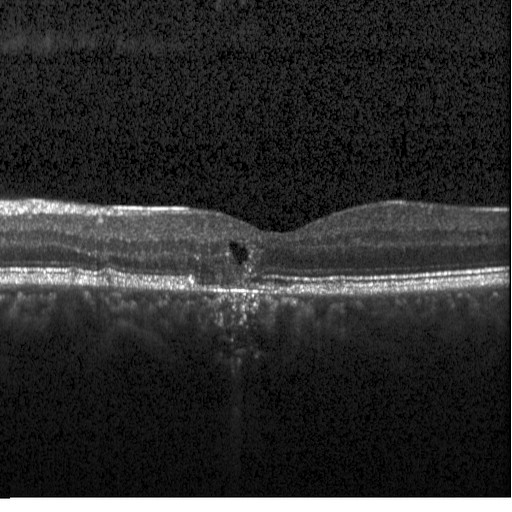

OCT B-scan; instrument: Heidelberg Spectralis
Finding: DME.